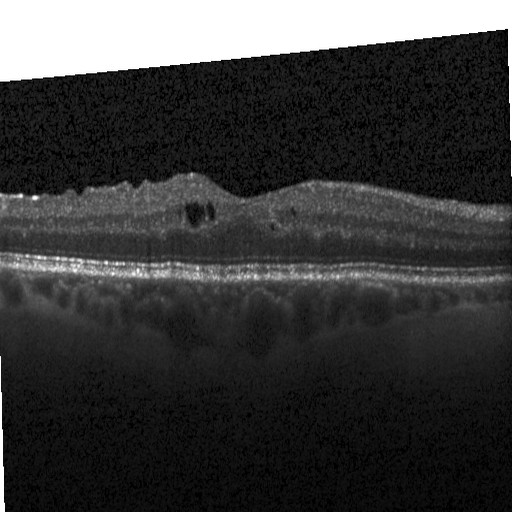
Dx: diabetic macular edema.